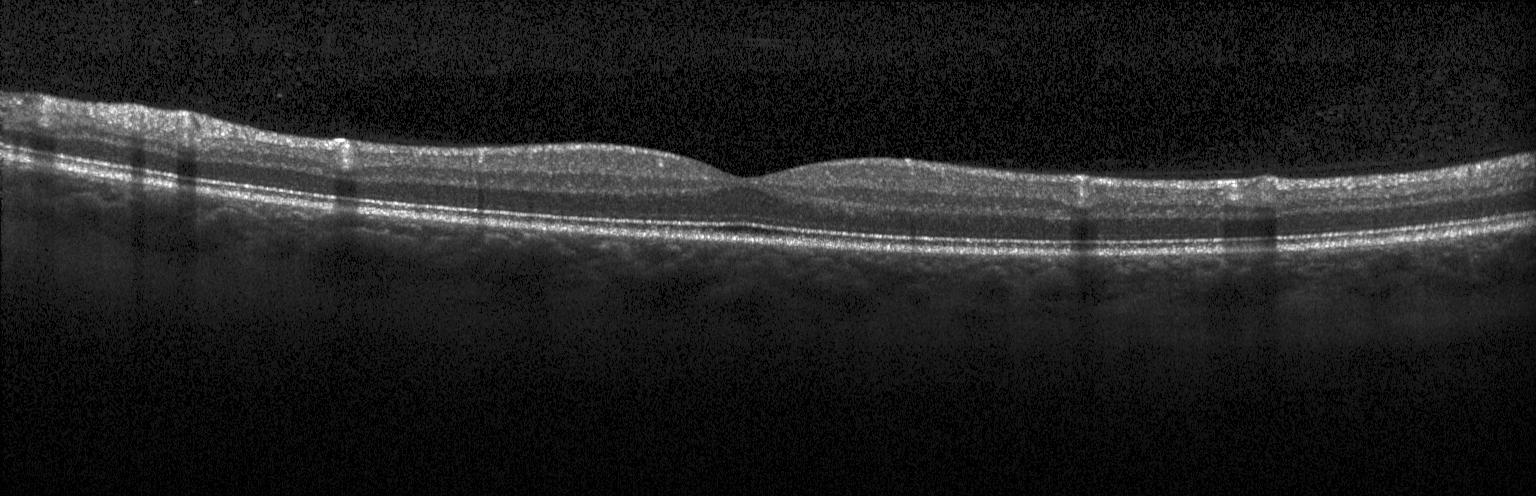

OCT line scan, spectral-domain optical coherence tomography, Heidelberg Spectralis OCT system, fovea-centered.
The scan shows no CNV, DME, or drusen.